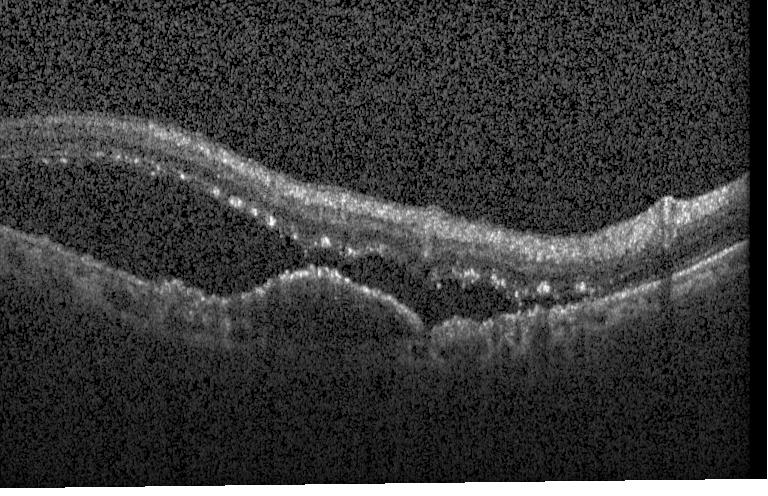

OCT B-scan showing choroidal neovascularization (CNV).